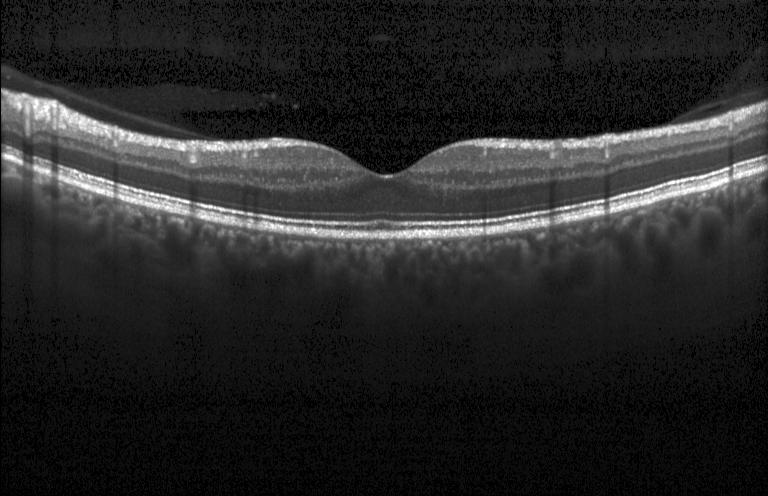

Optical coherence tomography B-scan.
Diagnosis: no choroidal neovascularization, diabetic macular edema, or drusen.